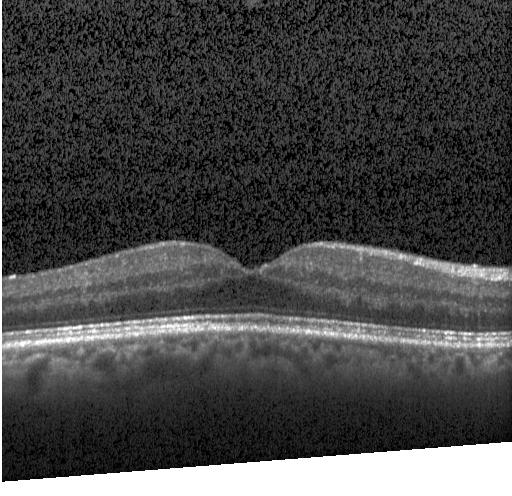 Spectral-domain OCT B-scan: no CNV, no DME, and no drusen.